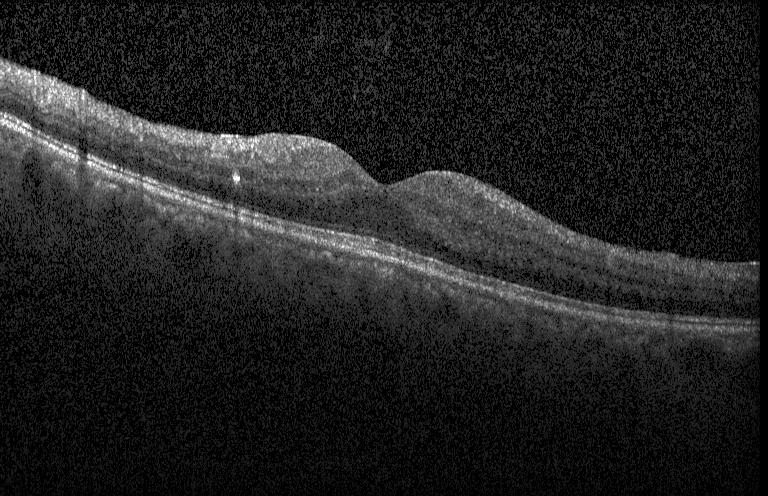
Finding: neither choroidal neovascularization, diabetic macular edema, nor drusen.